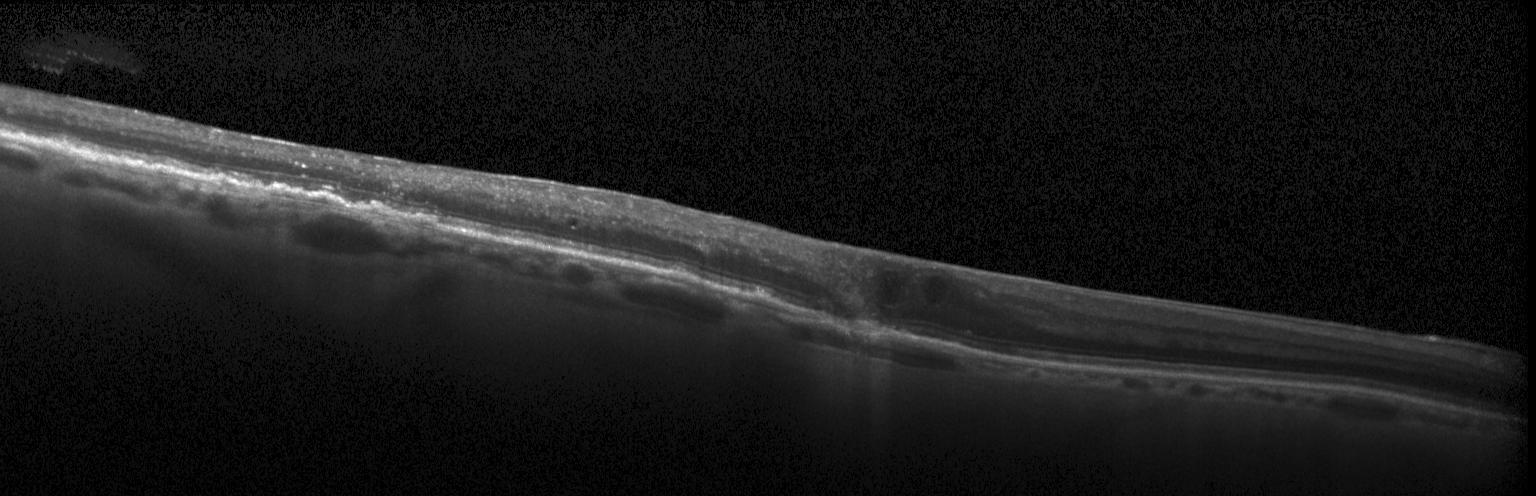 OCT B-scan.
This B-scan demonstrates choroidal neovascularization (CNV).